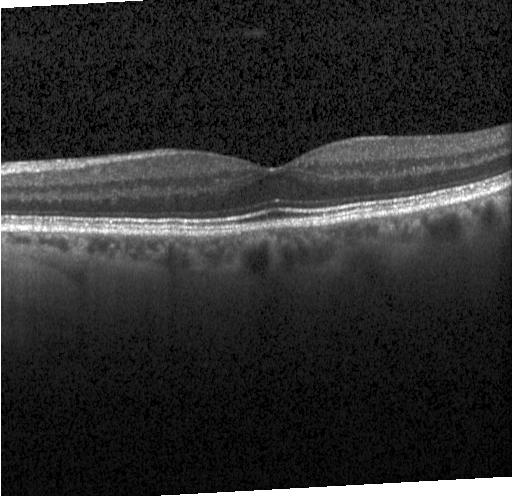 OCT line scan, spectral-domain optical coherence tomography — This B-scan demonstrates no choroidal neovascularization, no diabetic macular edema, and no drusen.